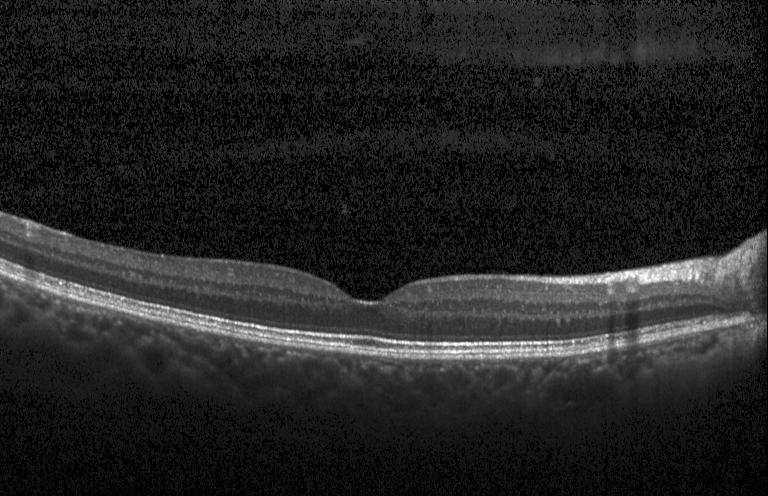
Optical coherence tomography B-scan. This B-scan demonstrates no choroidal neovascularization, diabetic macular edema, or drusen.